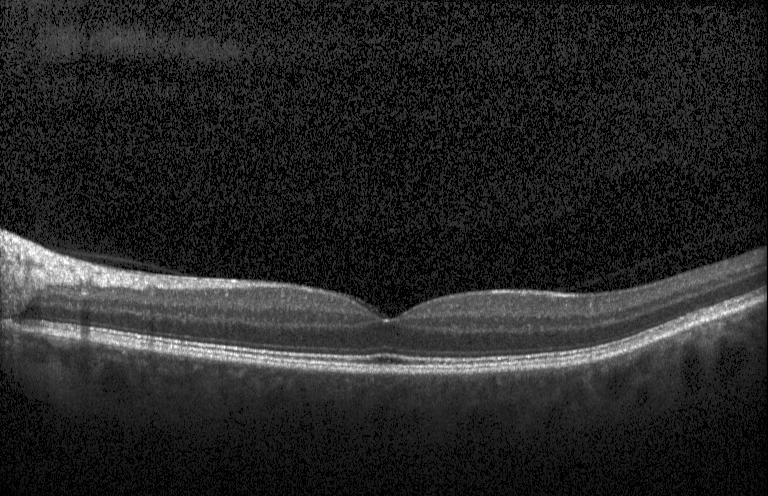

This B-scan demonstrates no choroidal neovascularization, no diabetic macular edema, and no drusen.